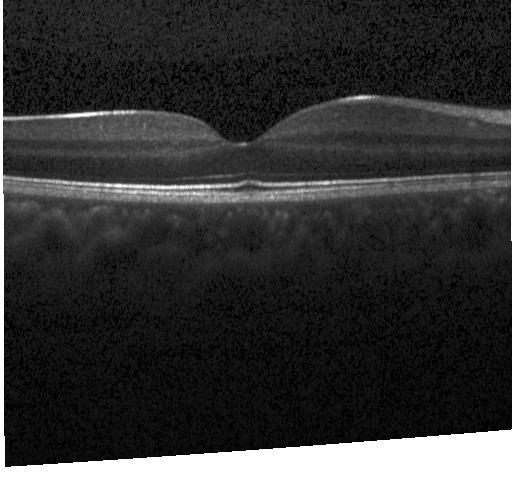

Spectral-domain optical coherence tomography, macular scan, acquired on a Heidelberg Spectralis, retinal OCT cross-section
No evidence of choroidal neovascularization, diabetic macular edema, or drusen.